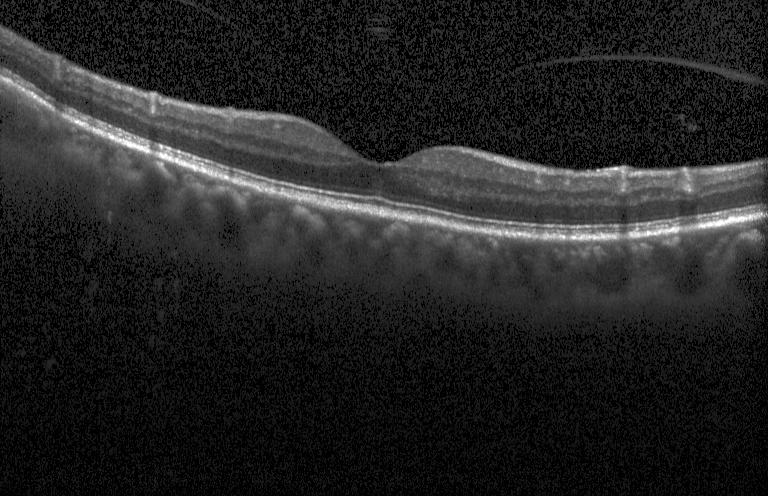
Retinal OCT B-scan. Acquired on a Heidelberg Spectralis. Horizontal scan through the fovea. Diagnosis: no choroidal neovascularization, diabetic macular edema, or drusen.